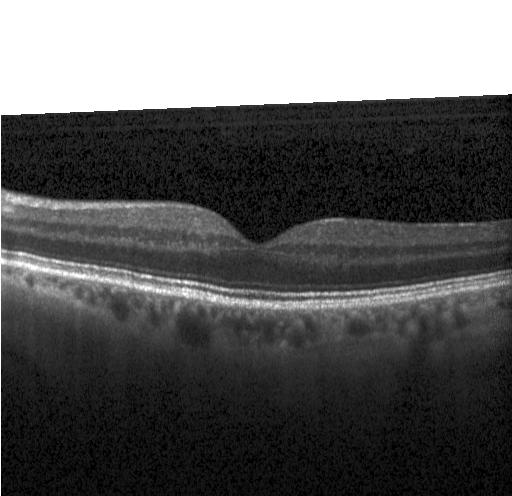

OCT line scan. Through the macula. Spectral-domain OCT.
Impression: neither choroidal neovascularization, diabetic macular edema, nor drusen.